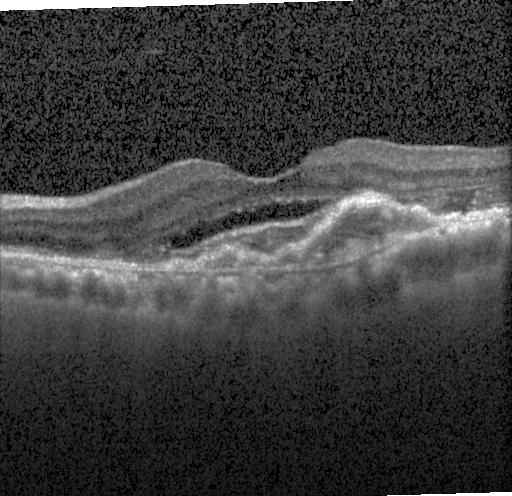
OCT B-scan.
Choroidal neovascularization.